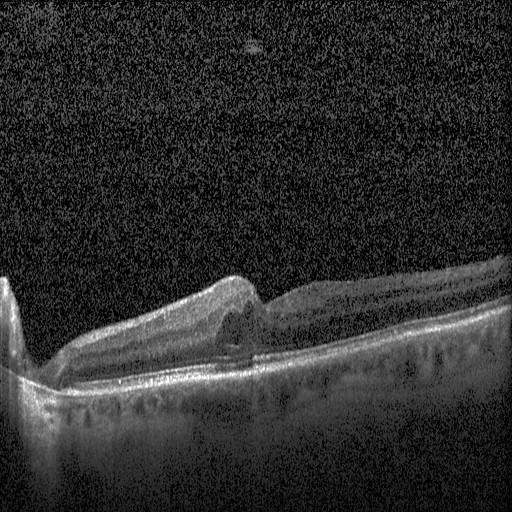
Through the macula; optical coherence tomography B-scan — Impression: DME.